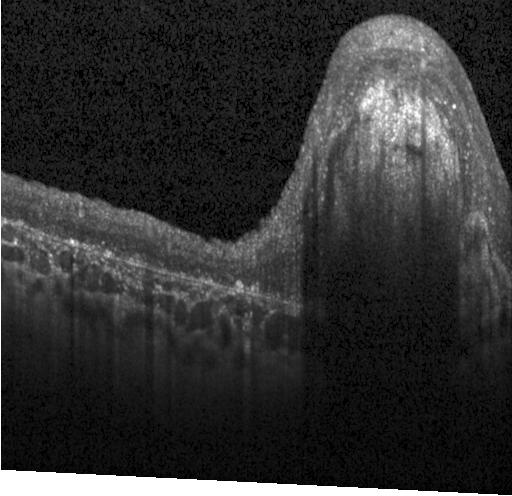

OCT B-scan.
Dx: a choroidal neovascular membrane.